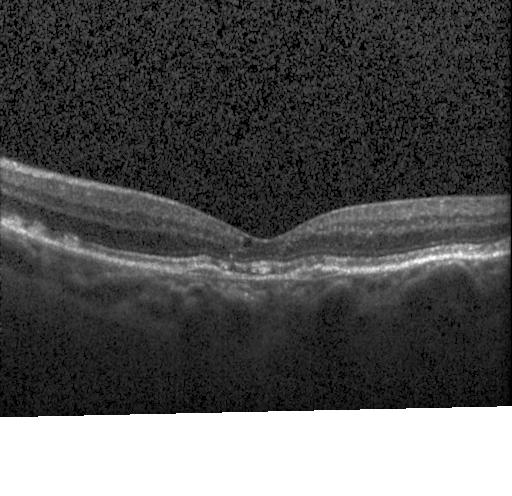

OCT B-scan showing a choroidal neovascular membrane.